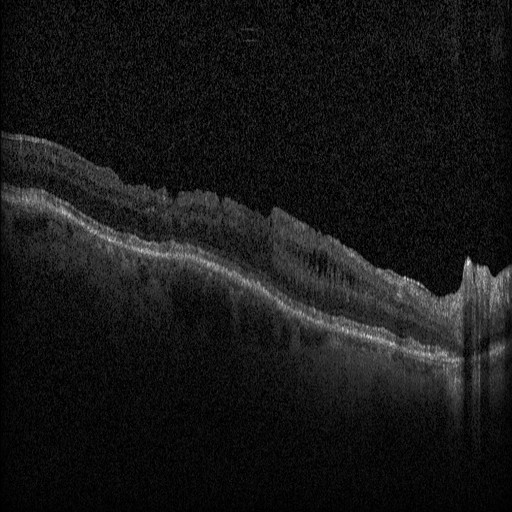

Centered on the fovea · optical coherence tomography scan
Finding: DME.